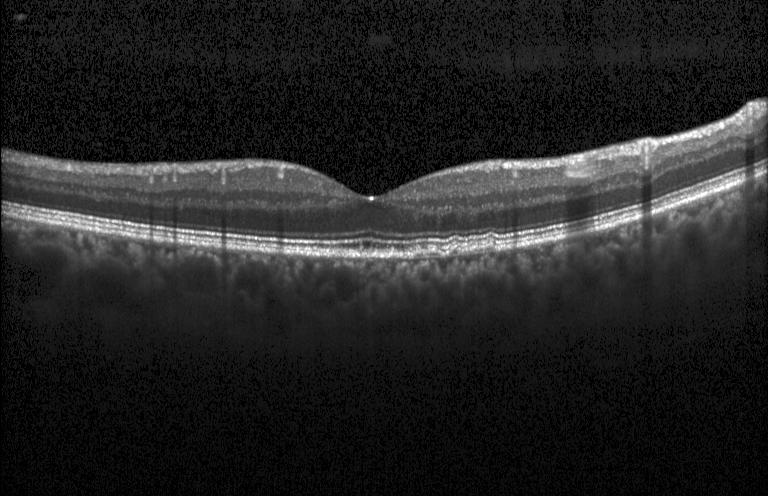

Macular OCT: sub-RPE drusenoid deposits.